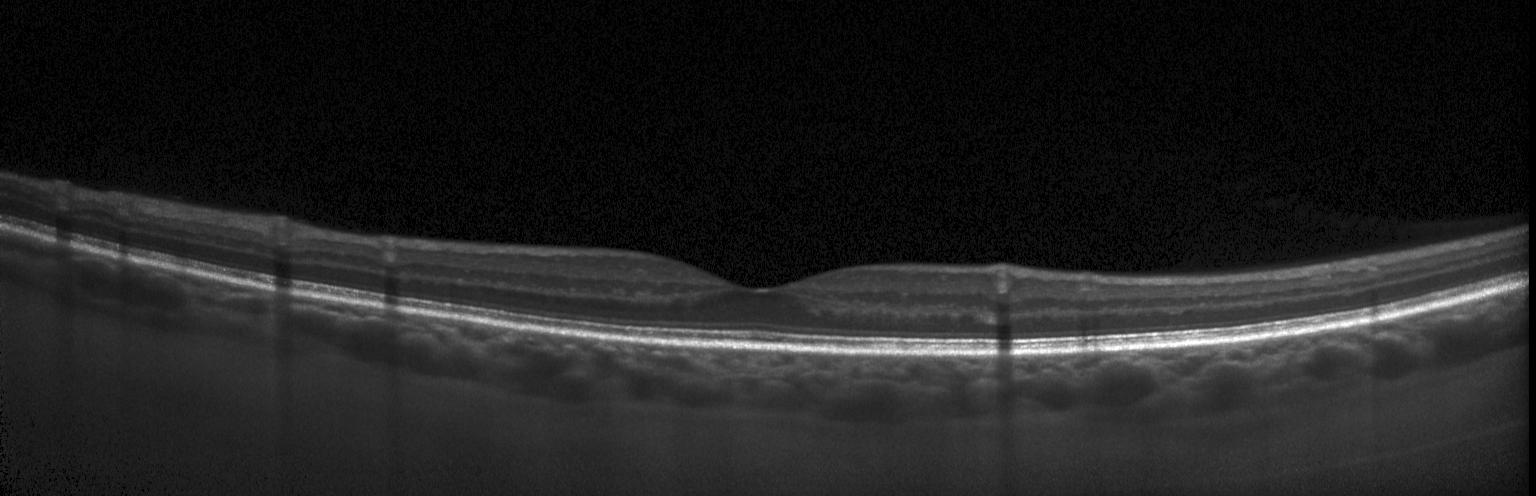

Optical coherence tomography B-scan · horizontal scan through the fovea
Macular OCT: no choroidal neovascularization, diabetic macular edema, or drusen.